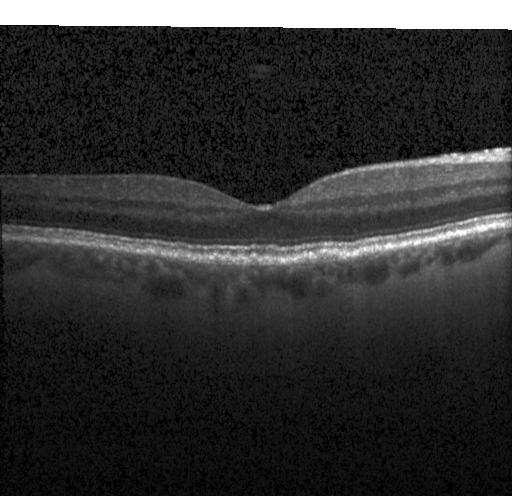

Retinal OCT cross-section, instrument: Heidelberg Spectralis, spectral-domain optical coherence tomography — This B-scan demonstrates multiple drusen.